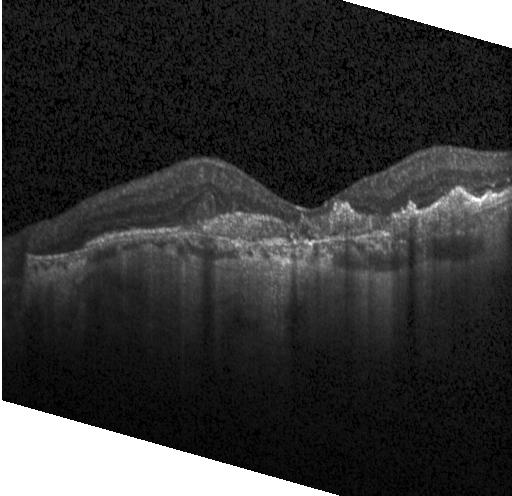

Optical coherence tomography scan, horizontal scan through the fovea. Impression: a choroidal neovascular membrane.